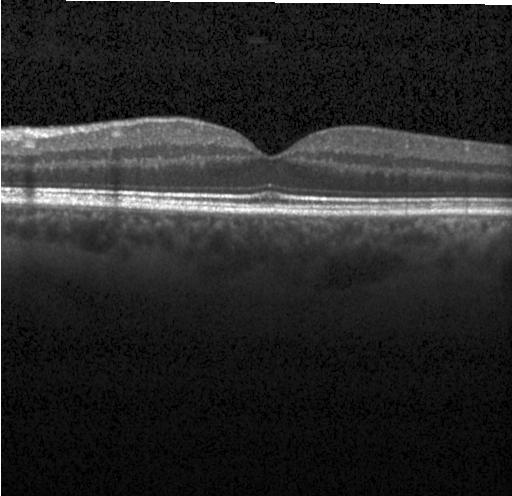

Impression: no evidence of CNV, DME, or drusen.